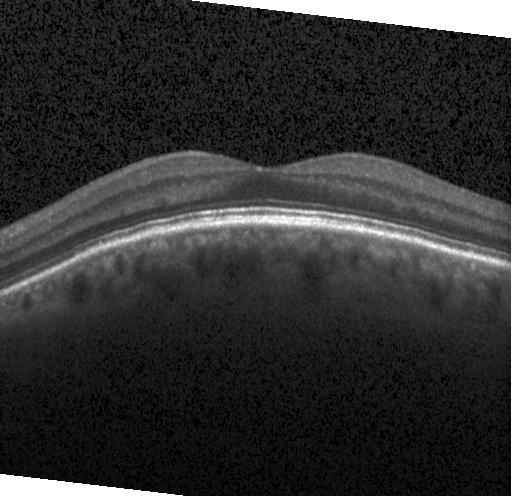

OCT scan showing no evidence of CNV, DME, or drusen.